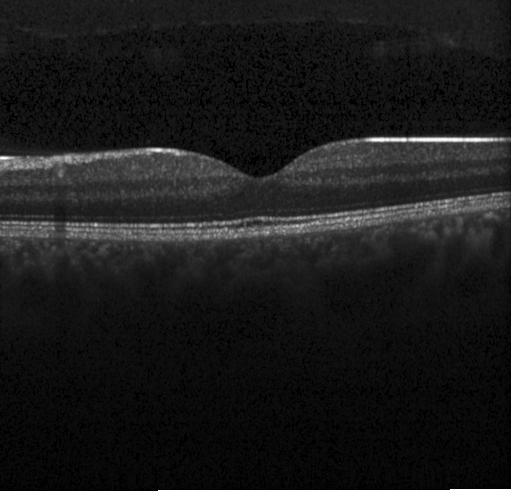
Macular scan · retinal OCT cross-section · Heidelberg Spectralis · spectral-domain optical coherence tomography.
This B-scan demonstrates no CNV, no DME, and no drusen.